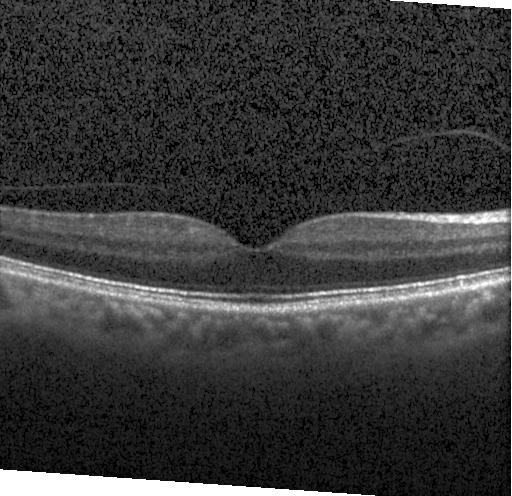

Retinal OCT cross-section showing neither CNV, DME, nor drusen.